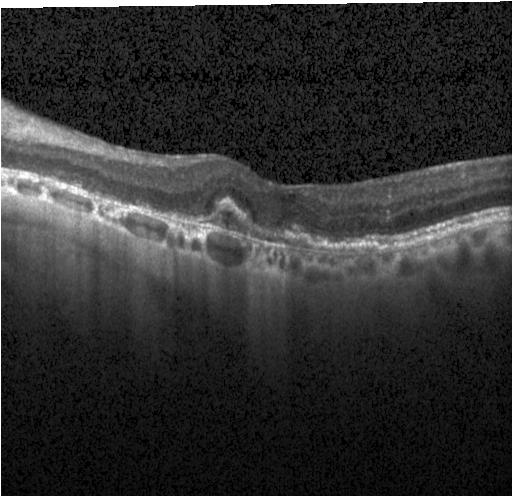 Retinal OCT cross-section showing choroidal neovascularization.